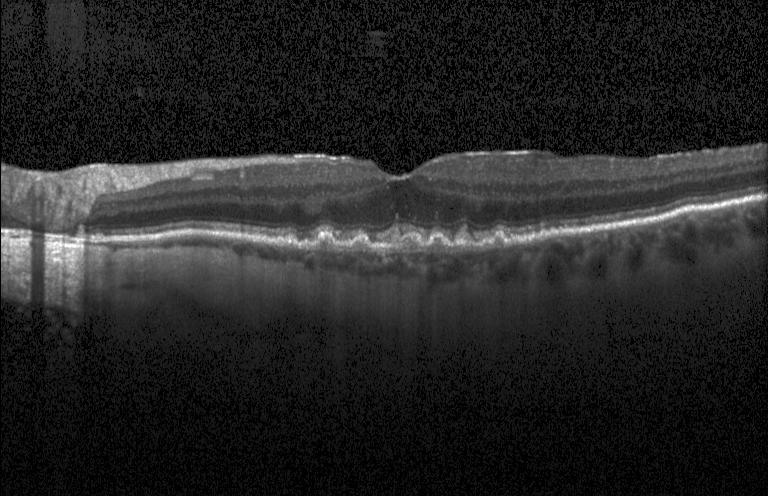

This B-scan demonstrates sub-RPE drusenoid deposits.